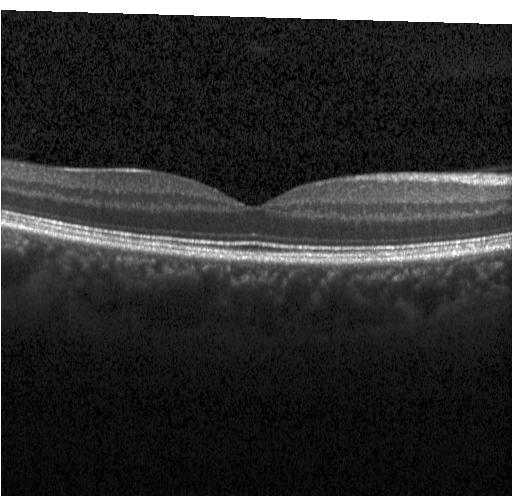 Heidelberg Spectralis OCT system · spectral-domain OCT · optical coherence tomography B-scan.
Neither choroidal neovascularization, diabetic macular edema, nor drusen.